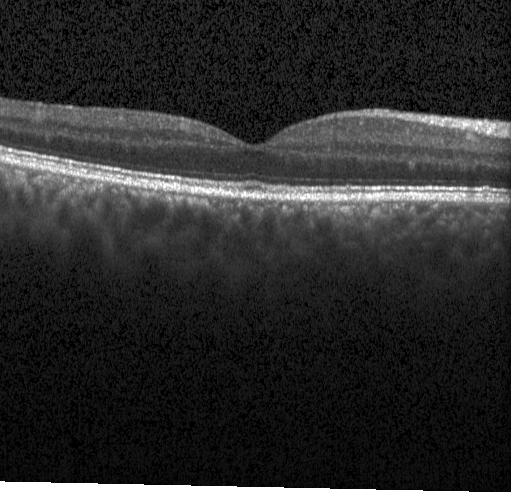

The scan shows no evidence of CNV, DME, or drusen.